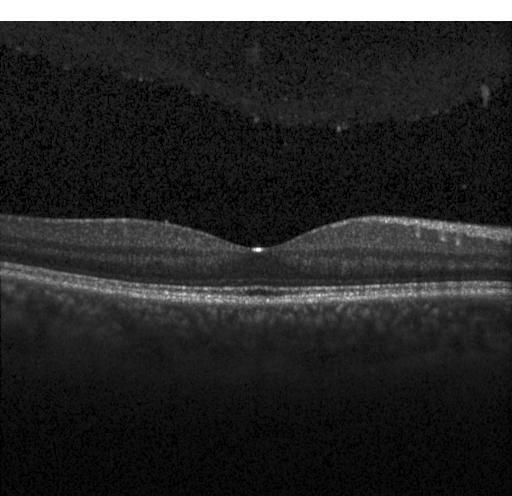

Macular OCT: no choroidal neovascularization, no diabetic macular edema, and no drusen.